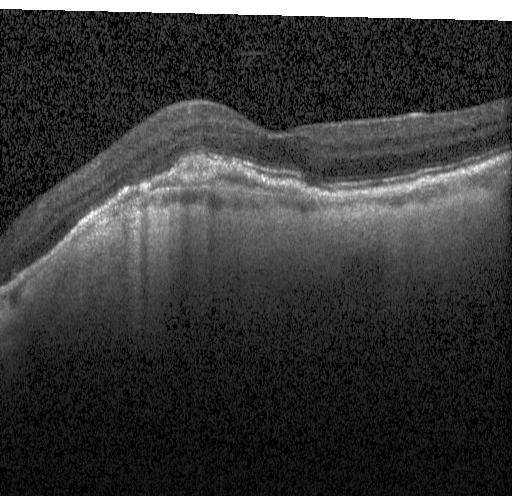
Centered on the fovea; OCT B-scan; spectral-domain OCT; acquired on a Heidelberg Spectralis
This B-scan demonstrates a choroidal neovascular membrane.